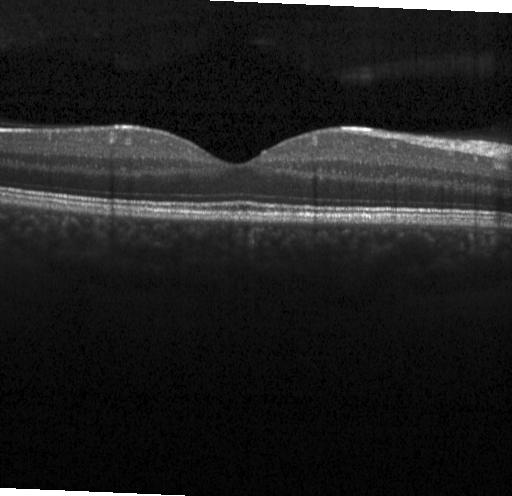

Retinal OCT cross-section showing neither choroidal neovascularization, diabetic macular edema, nor drusen.